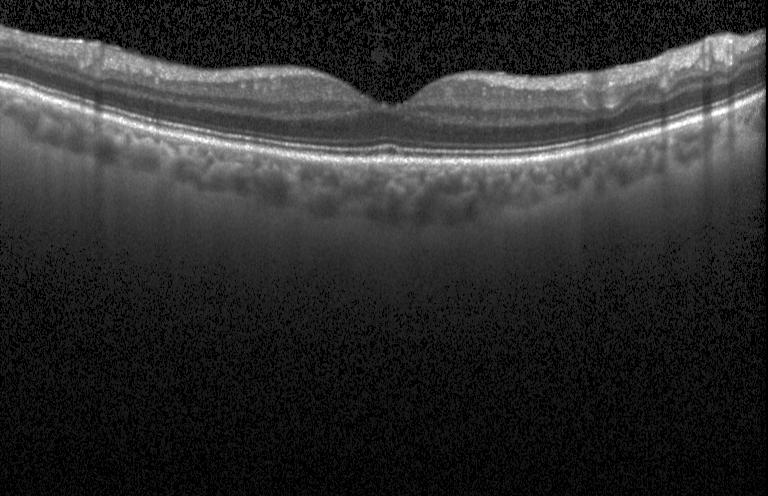
Spectral-domain optical coherence tomography; Heidelberg Spectralis OCT system; optical coherence tomography scan.
Dx: no CNV, DME, or drusen.